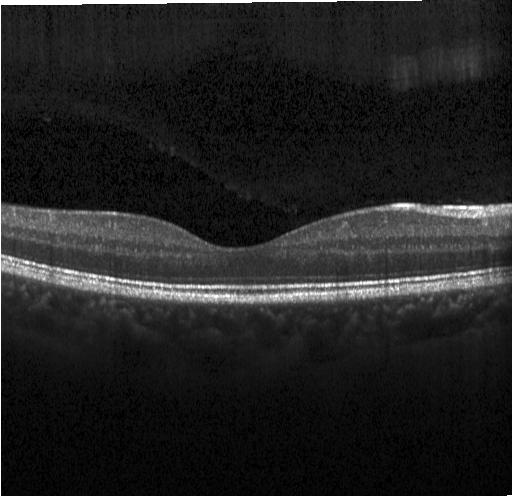 Impression: neither CNV, DME, nor drusen.